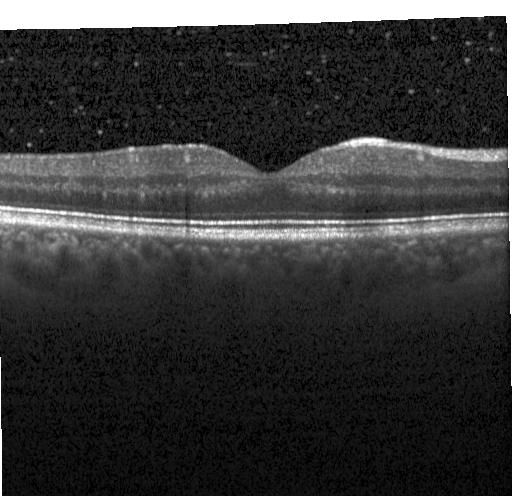

Impression: neither choroidal neovascularization, diabetic macular edema, nor drusen.